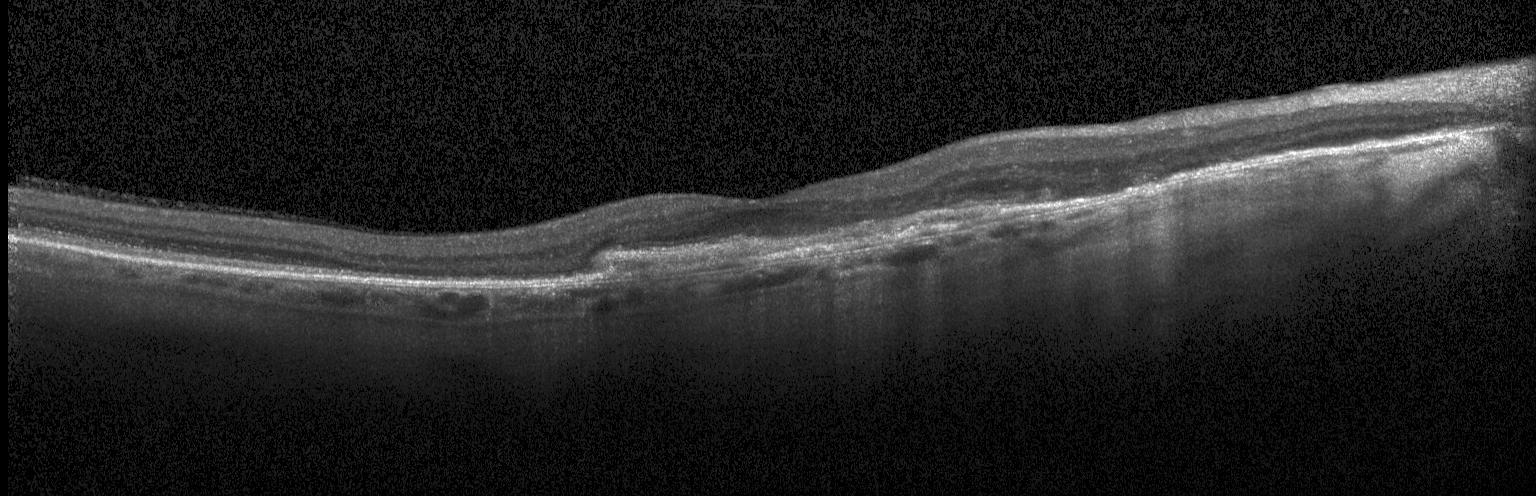

The scan shows a choroidal neovascular membrane.